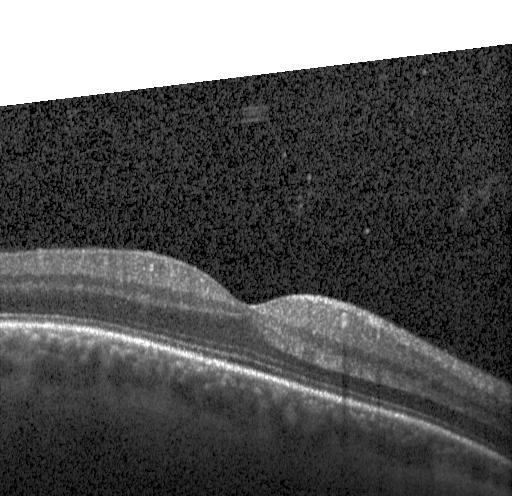 Impression: neither CNV, DME, nor drusen.